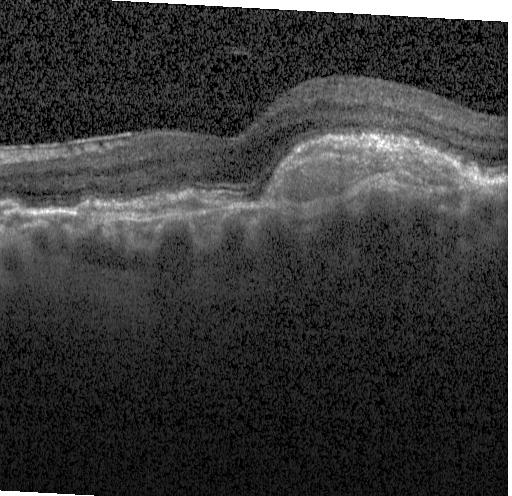 SD-OCT · horizontal scan through the fovea · retinal OCT cross-section. Macular OCT: CNV.